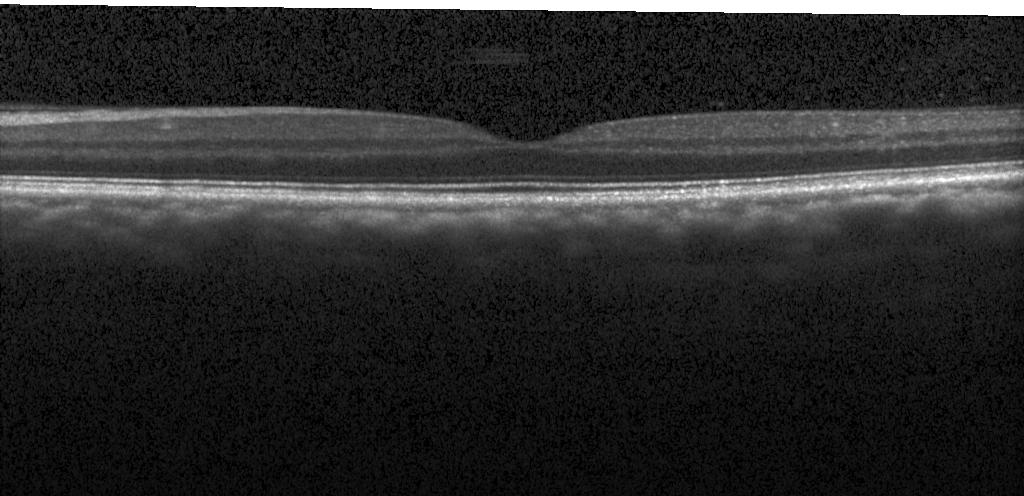

Spectral-domain optical coherence tomography. OCT B-scan. Horizontal scan through the fovea. Instrument: Heidelberg Spectralis.
Impression: neither choroidal neovascularization, diabetic macular edema, nor drusen.